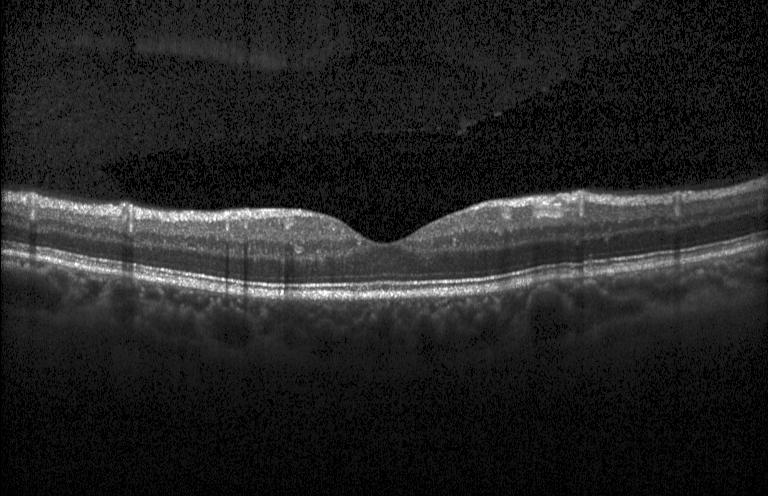
Macular OCT demonstrating no evidence of CNV, DME, or drusen.